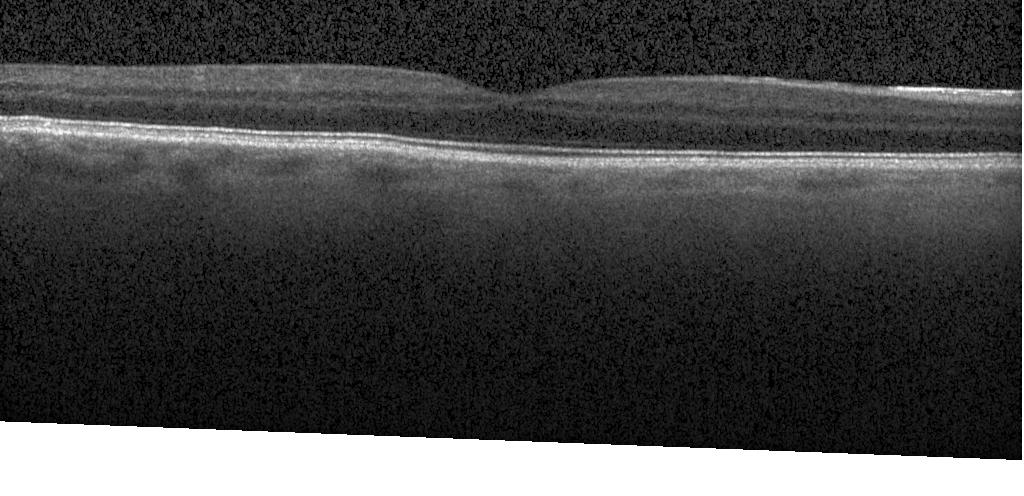

Diagnosis: no CNV, no DME, and no drusen.